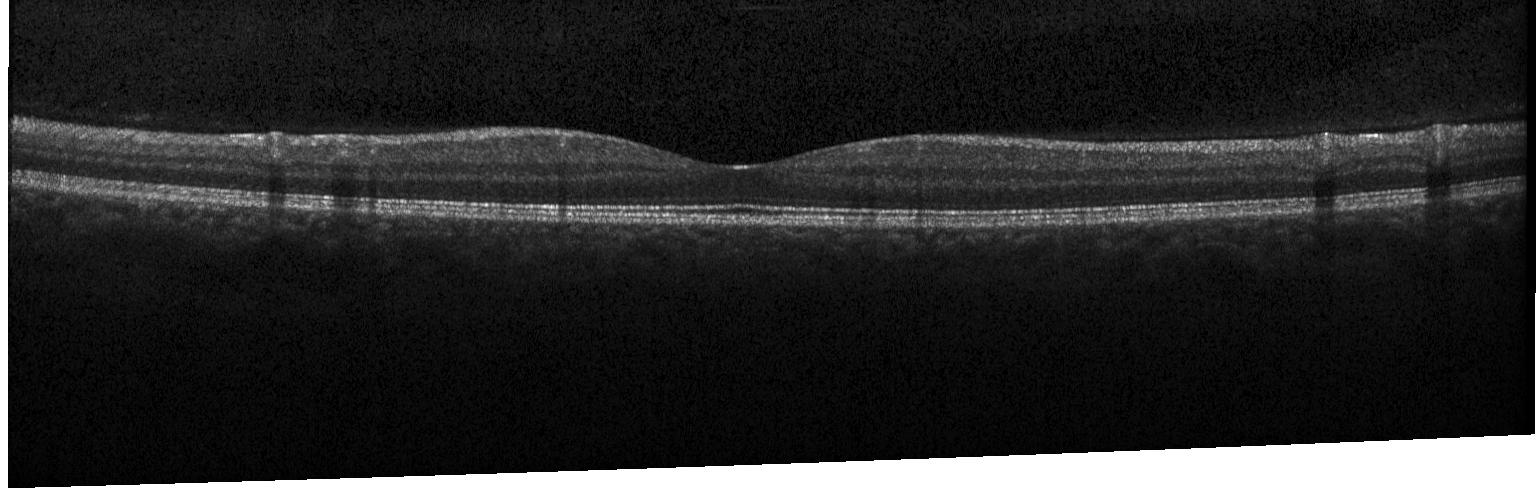
Instrument: Heidelberg Spectralis · SD-OCT · retinal OCT B-scan
Impression: no choroidal neovascularization, no diabetic macular edema, and no drusen.